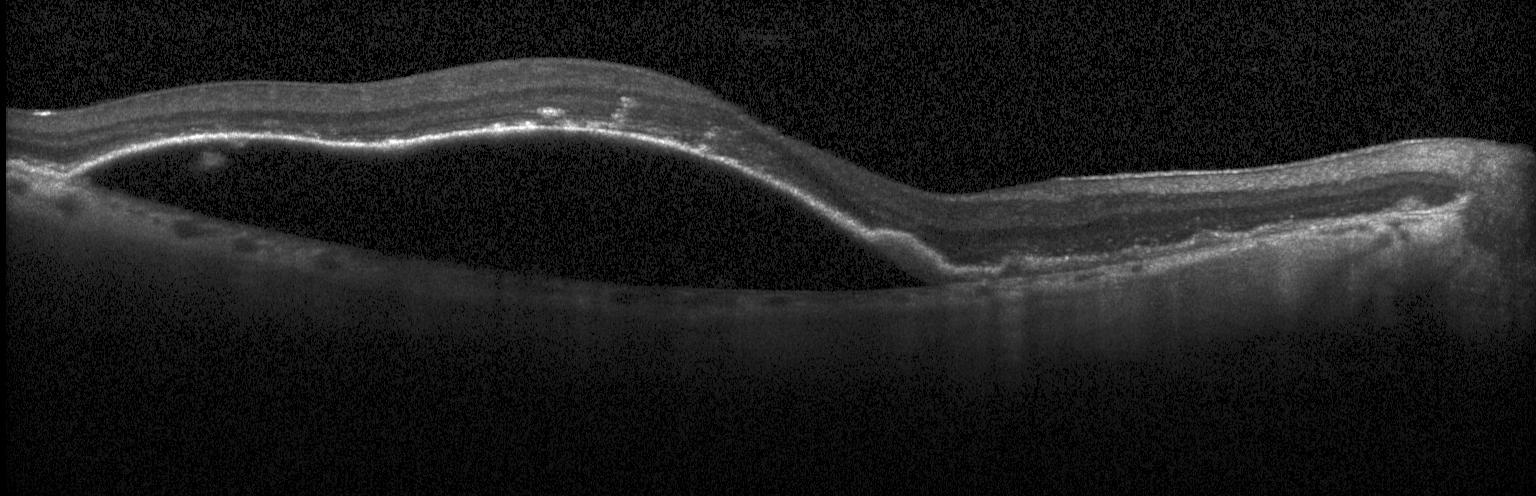
Optical coherence tomography B-scan; SD-OCT. Assessment: CNV.